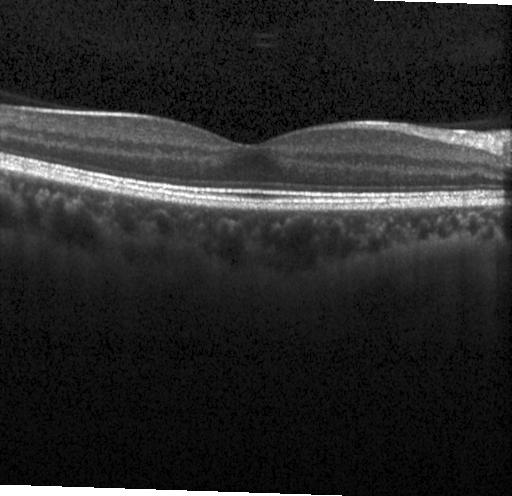 OCT B-scan; through the macula; SD-OCT; instrument: Heidelberg Spectralis. Macular OCT: no choroidal neovascularization, no diabetic macular edema, and no drusen.